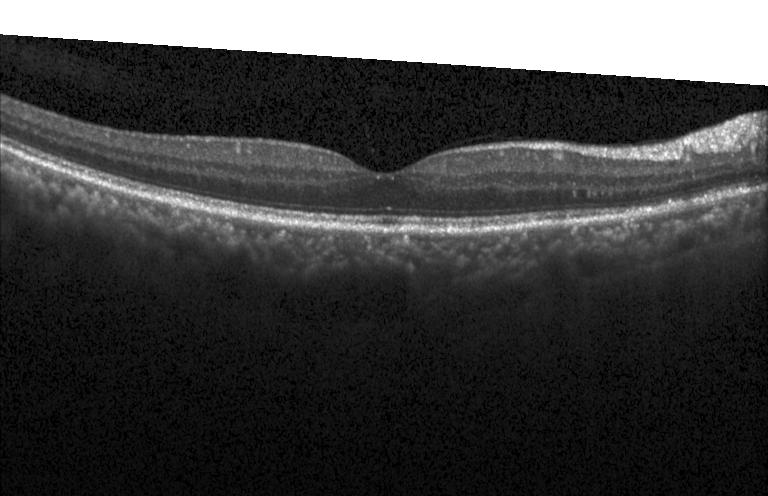
Optical coherence tomography scan. Heidelberg Spectralis OCT system. Horizontal scan through the fovea. Spectral-domain OCT — OCT finding: no evidence of CNV, DME, or drusen.